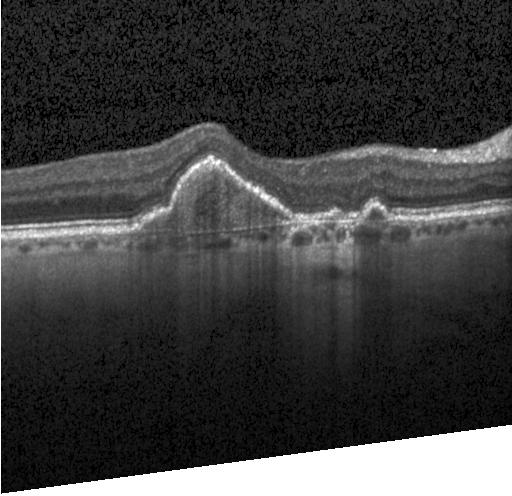
OCT scan showing a choroidal neovascular membrane.